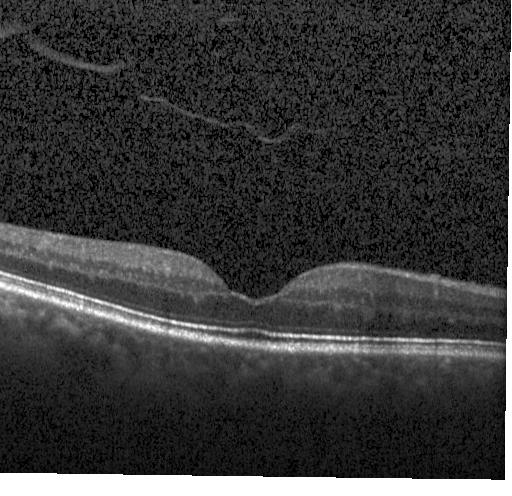 Optical coherence tomography scan. Impression: no evidence of choroidal neovascularization, diabetic macular edema, or drusen.